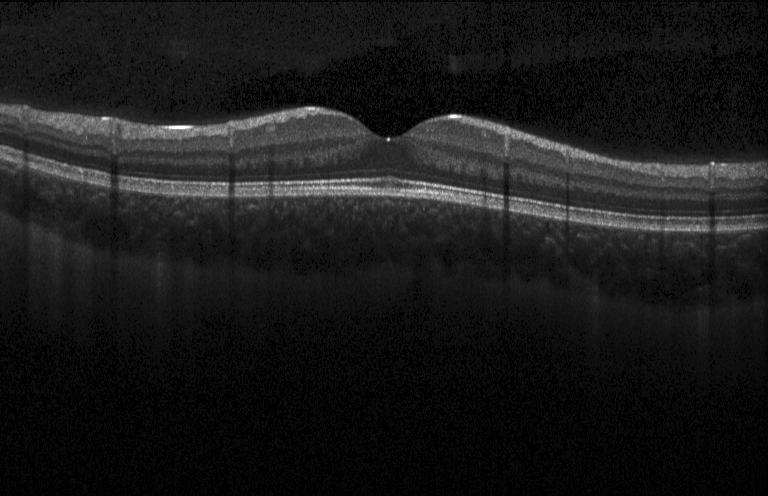

Spectral-domain OCT B-scan: neither choroidal neovascularization, diabetic macular edema, nor drusen.